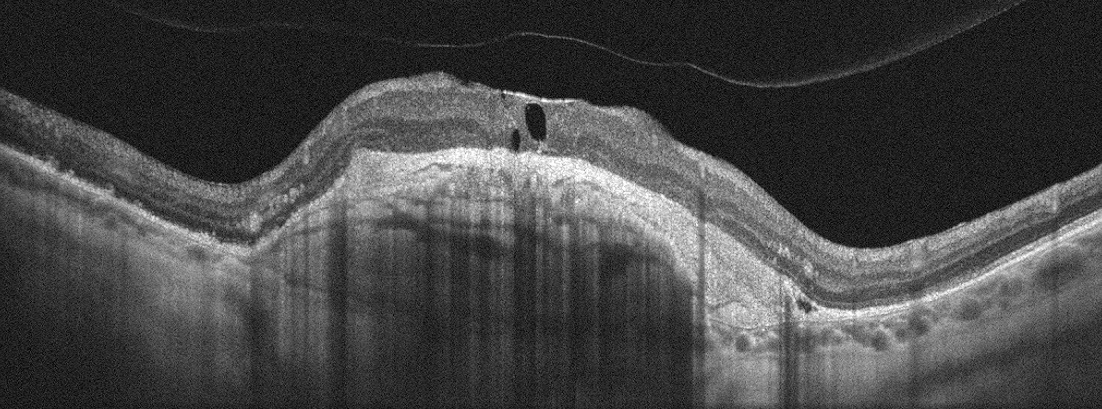 The scan shows age-related macular degeneration.